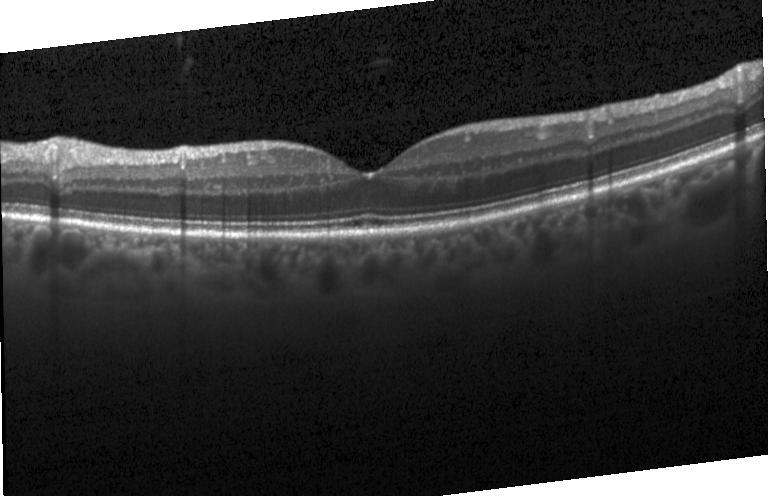
Through the macula, OCT line scan, instrument: Heidelberg Spectralis. No evidence of choroidal neovascularization, diabetic macular edema, or drusen.